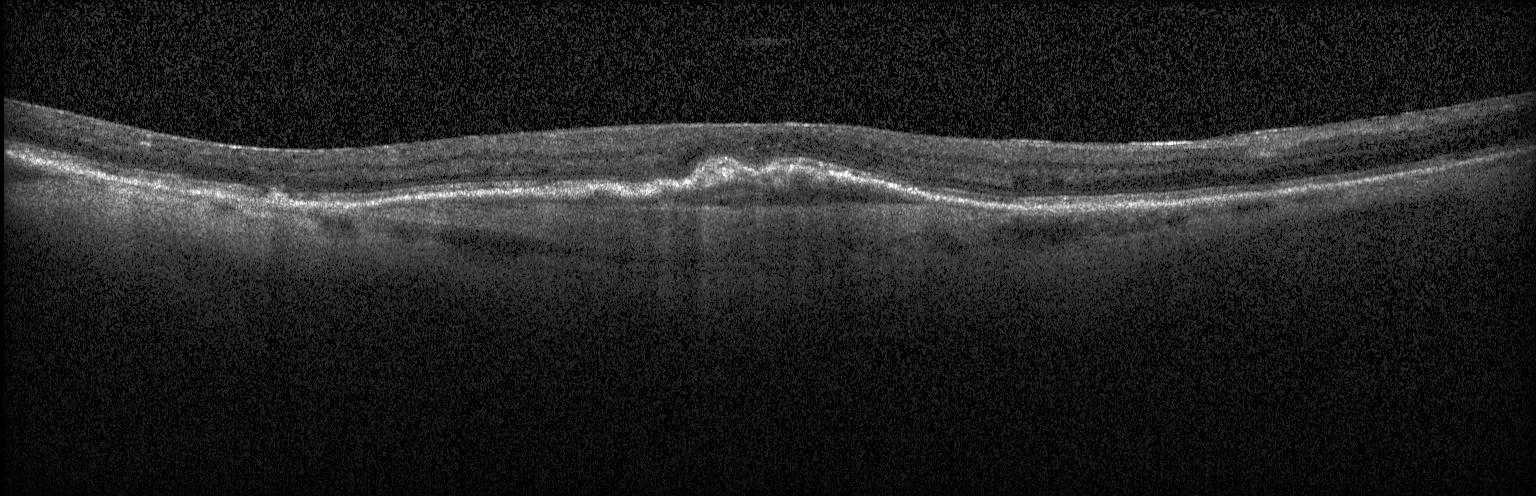 Retinal OCT cross-section showing choroidal neovascularization.